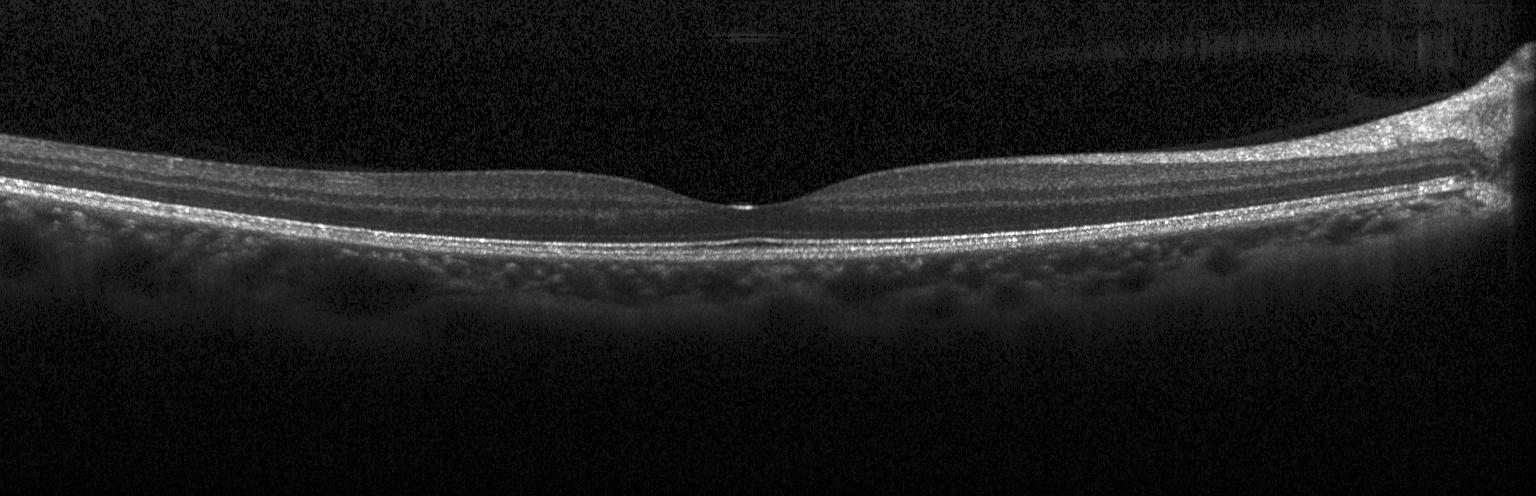 OCT B-scan · SD-OCT · Heidelberg Spectralis — Finding: no choroidal neovascularization, diabetic macular edema, or drusen.